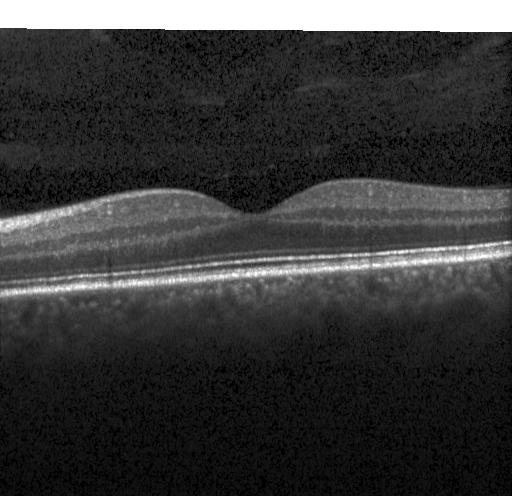

OCT finding: no choroidal neovascularization, diabetic macular edema, or drusen.